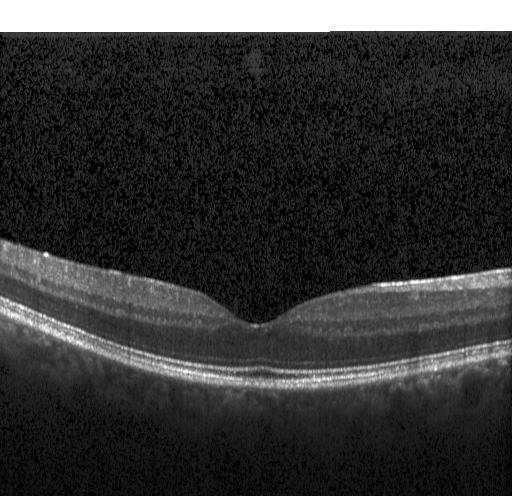

Heidelberg Spectralis; spectral-domain OCT; OCT line scan; through the macula.
No choroidal neovascularization, diabetic macular edema, or drusen.